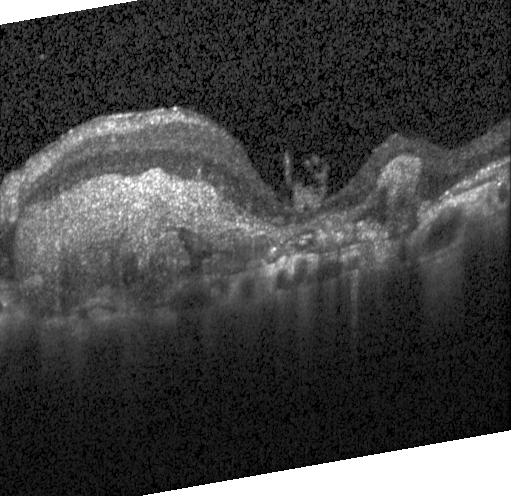 Retinal OCT cross-section; Heidelberg Spectralis. Diagnosis: a choroidal neovascular membrane.